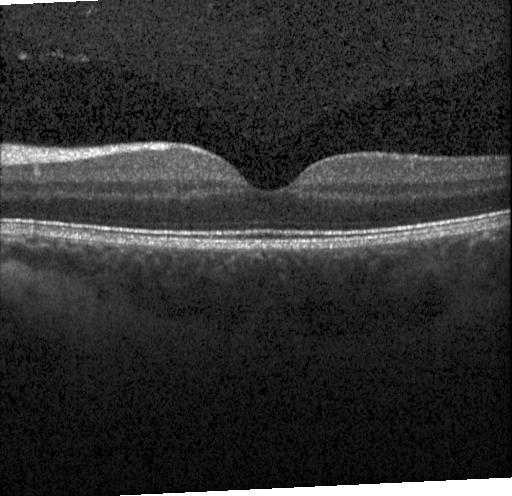 Optical coherence tomography B-scan, fovea-centered, SD-OCT, Heidelberg Spectralis — Diagnosis: no choroidal neovascularization, diabetic macular edema, or drusen.